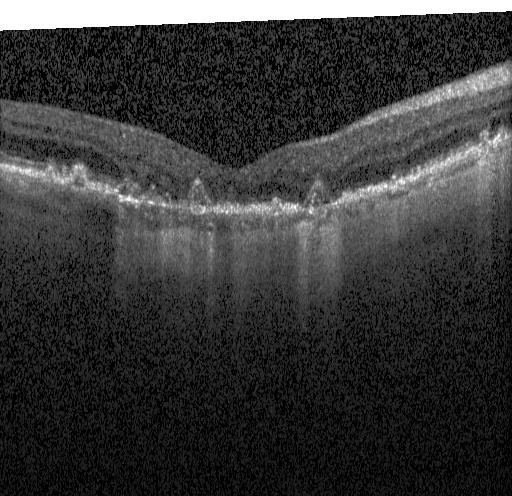 Dx: choroidal neovascularization (CNV).